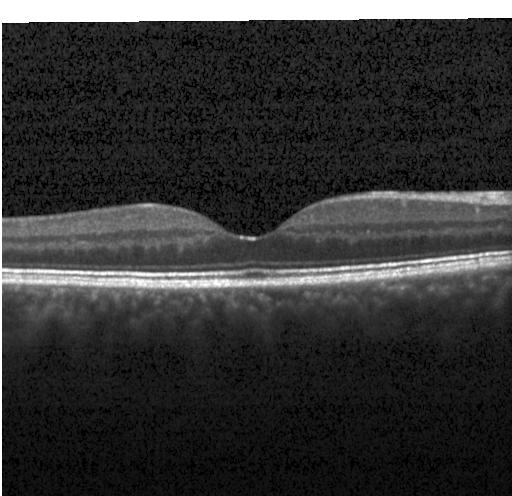
Horizontal scan through the fovea. Heidelberg Spectralis OCT system. OCT B-scan — Assessment: no choroidal neovascularization, no diabetic macular edema, and no drusen.